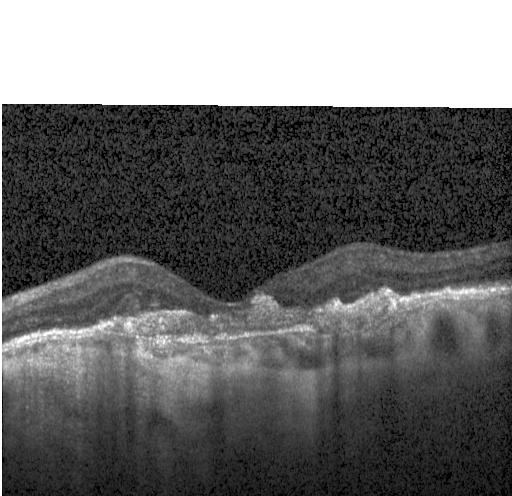
OCT B-scan. Centered on the fovea. Spectral-domain optical coherence tomography. Heidelberg Spectralis.
Finding: choroidal neovascularization (CNV).